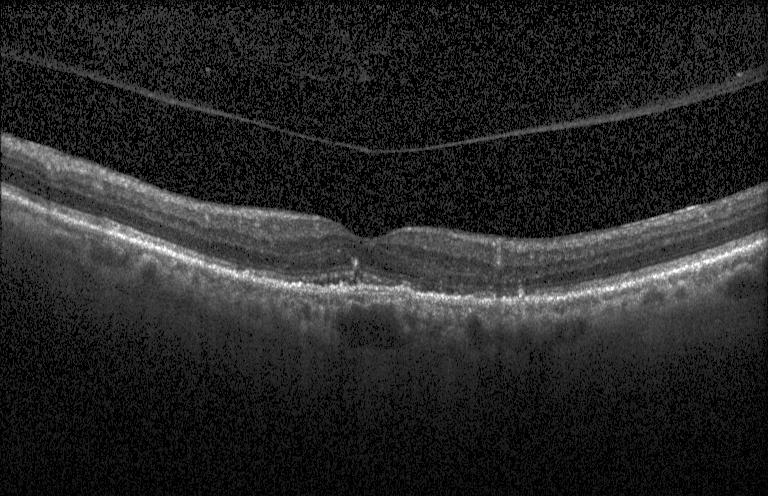

Centered on the fovea; instrument: Heidelberg Spectralis; OCT line scan; spectral-domain OCT
Impression: a choroidal neovascular membrane.